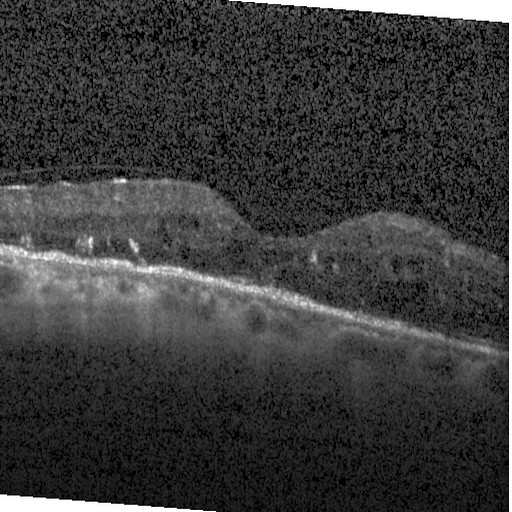 Fovea-centered; Heidelberg Spectralis; SD-OCT; optical coherence tomography scan — Diagnosis: diabetic macular edema (DME).